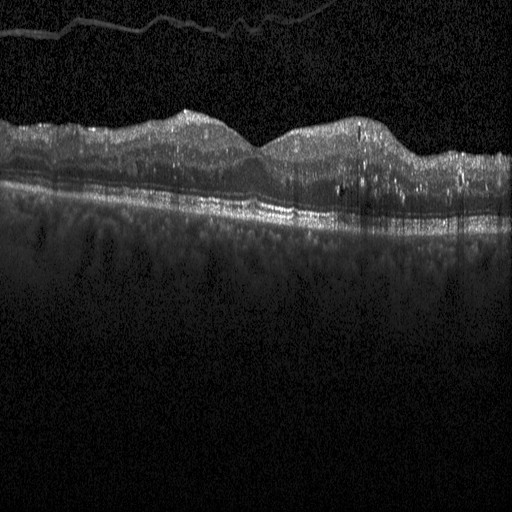 Finding: DME.